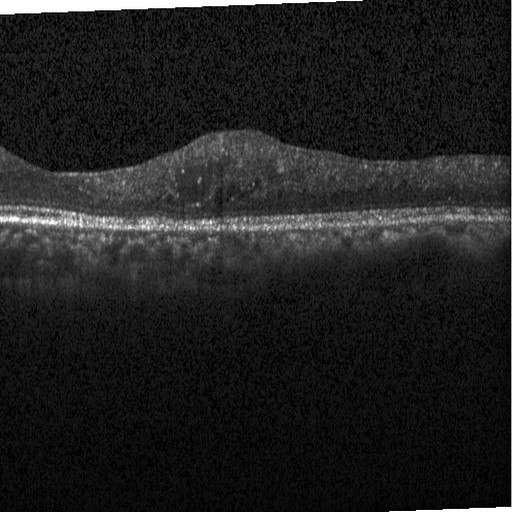
Centered on the fovea. OCT B-scan. Instrument: Heidelberg Spectralis. Spectral-domain OCT — The scan shows DME.